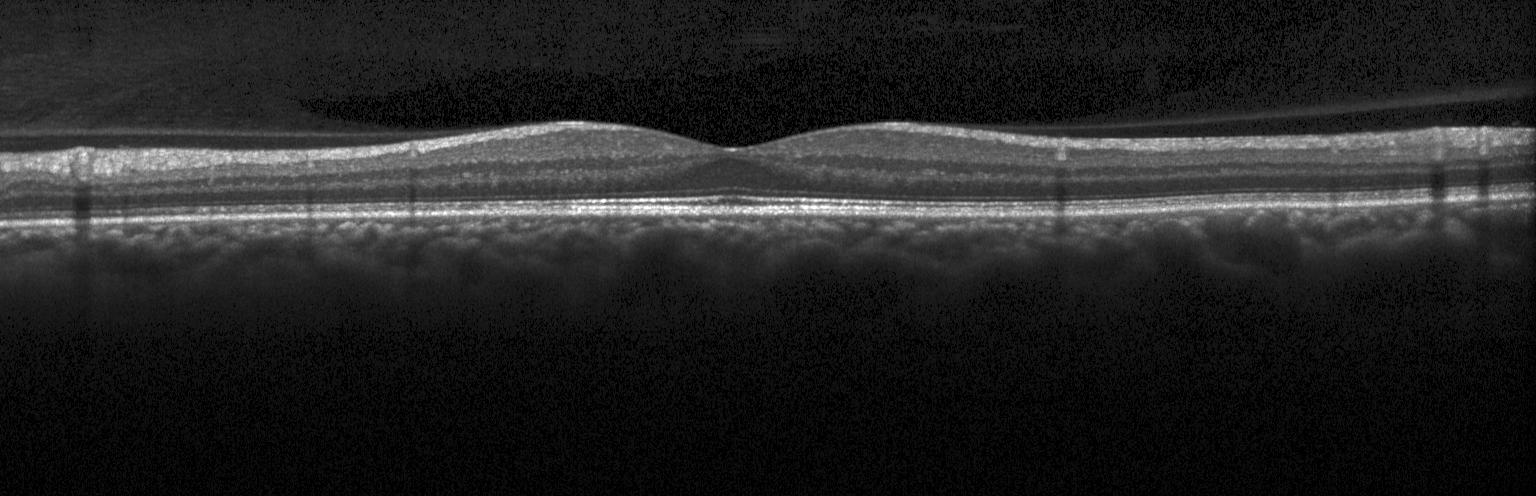 Centered on the fovea. Instrument: Heidelberg Spectralis. OCT B-scan
Finding: no choroidal neovascularization, diabetic macular edema, or drusen.